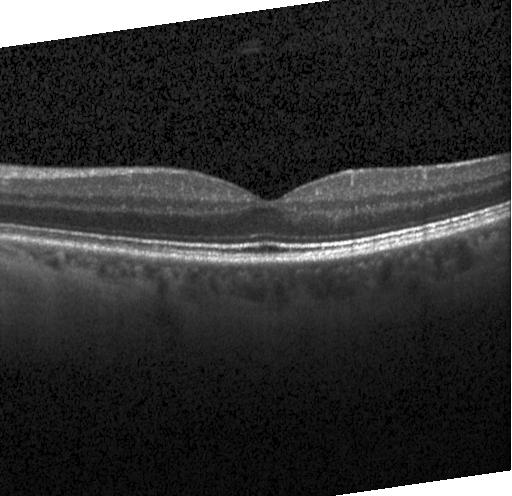 Optical coherence tomography scan
Impression: no evidence of choroidal neovascularization, diabetic macular edema, or drusen.